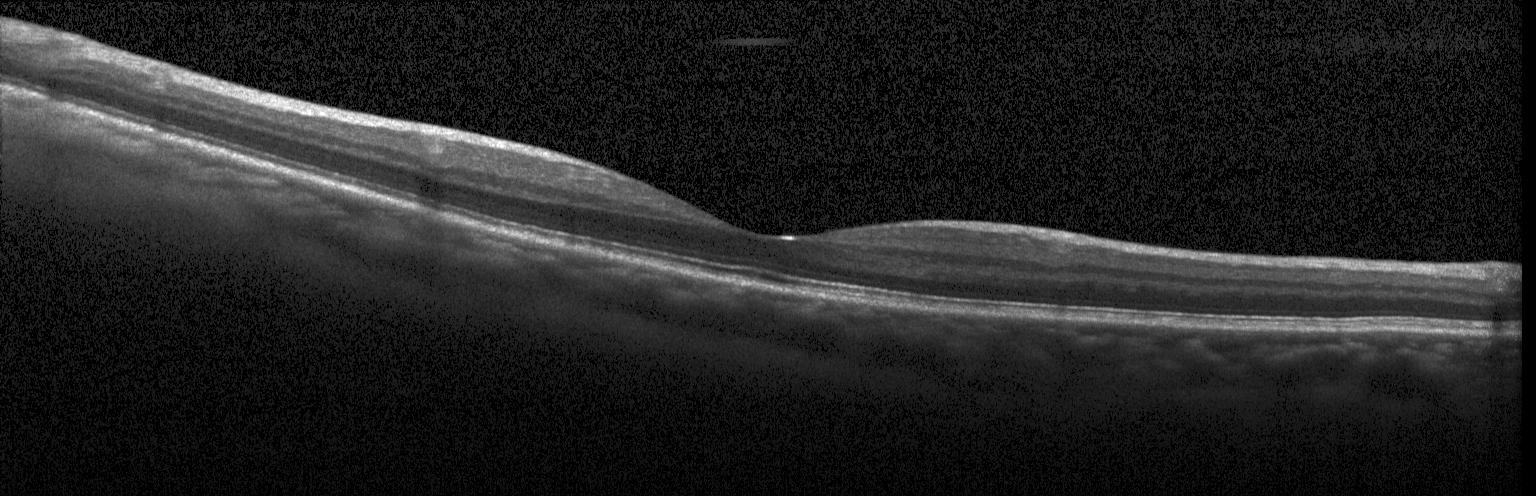 Optical coherence tomography B-scan — Finding: no choroidal neovascularization, diabetic macular edema, or drusen.